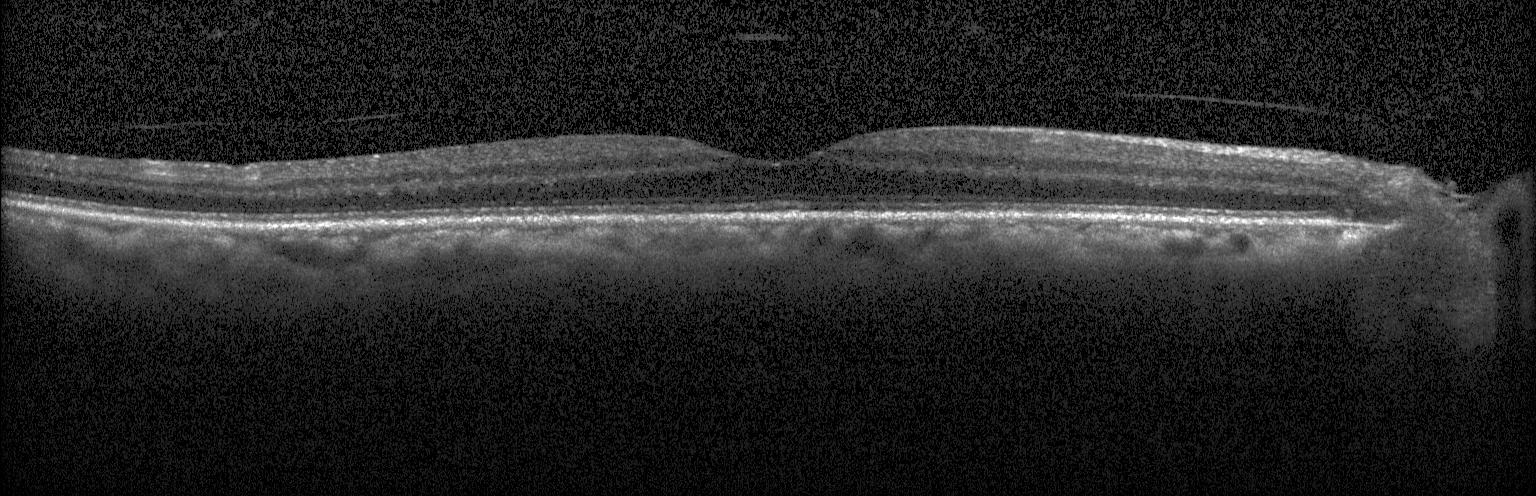
Retinal OCT cross-section. Diagnosis: neither CNV, DME, nor drusen.